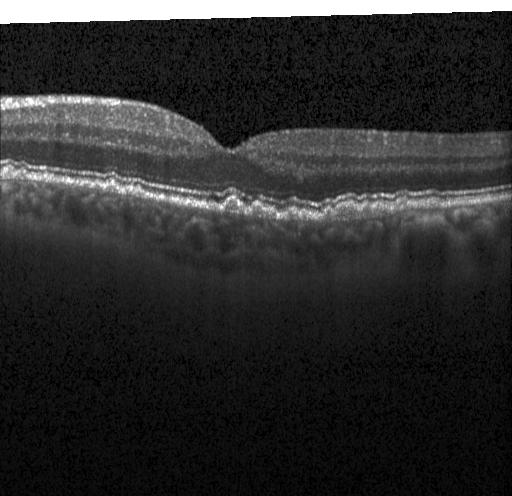

OCT line scan
OCT finding: drusen.